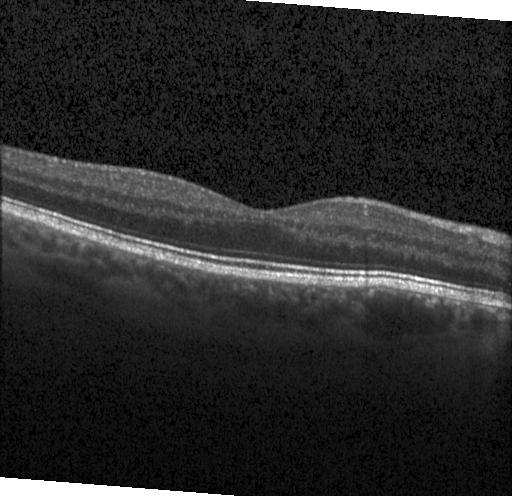
Retinal OCT cross-section.
This B-scan demonstrates no evidence of CNV, DME, or drusen.